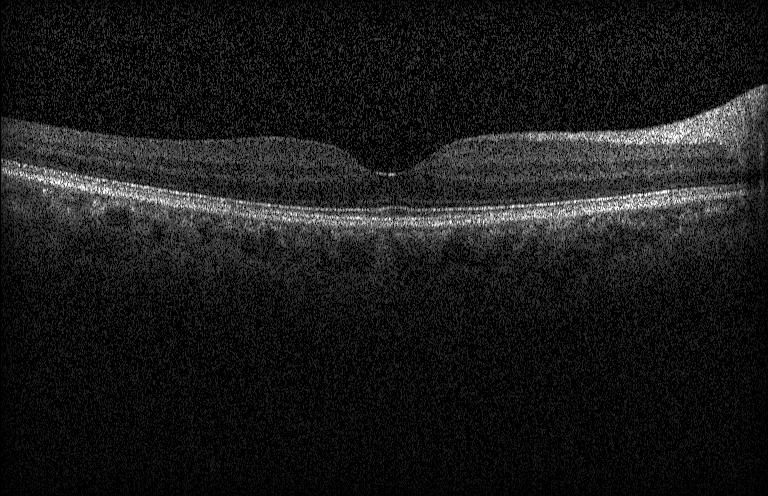
Optical coherence tomography scan — Assessment: no choroidal neovascularization, no diabetic macular edema, and no drusen.